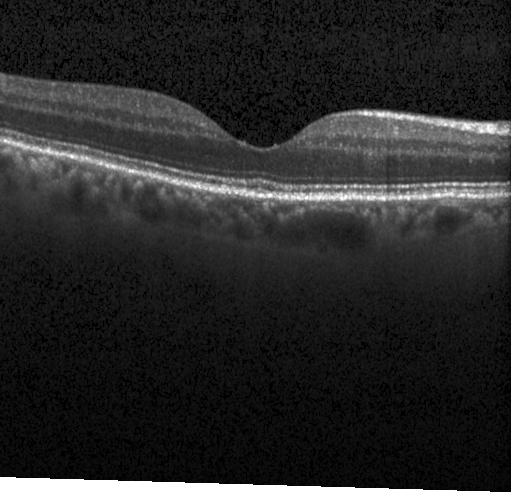
Acquired on a Heidelberg Spectralis, fovea-centered, SD-OCT, optical coherence tomography scan.
Diagnosis: no choroidal neovascularization, no diabetic macular edema, and no drusen.